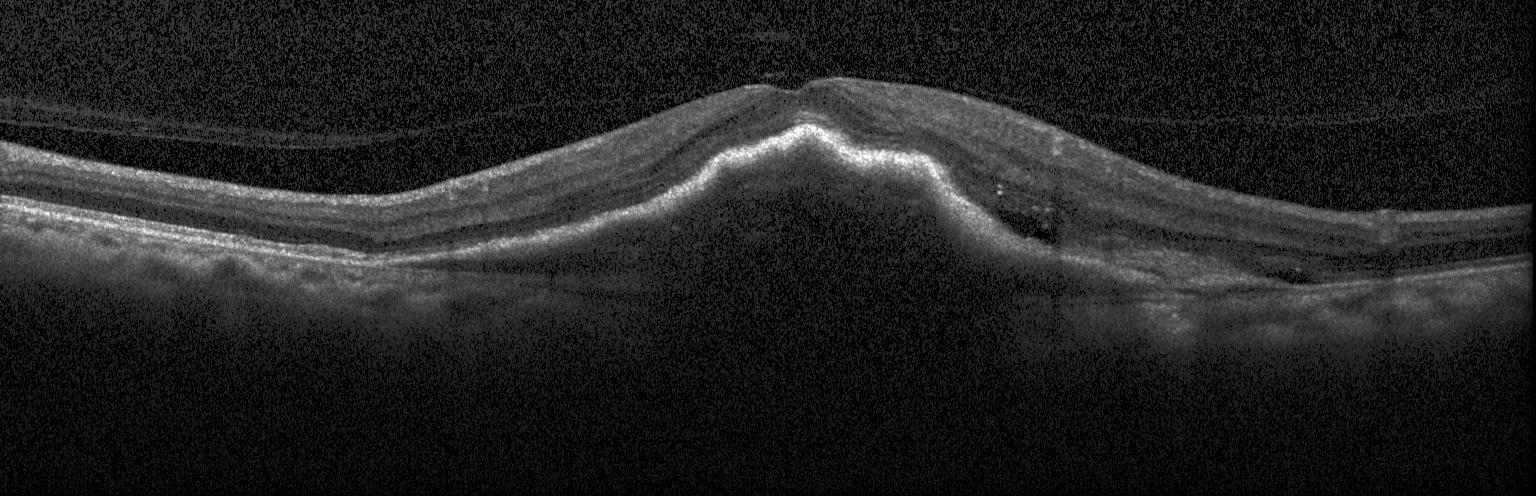

Retinal OCT B-scan, spectral-domain optical coherence tomography.
Impression: choroidal neovascularization.